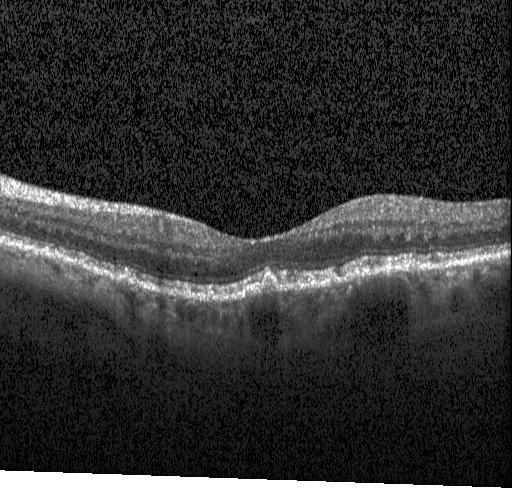 Finding: multiple drusen.